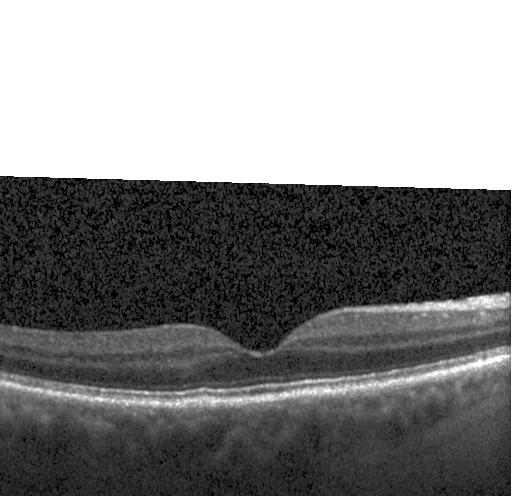
OCT B-scan, macular scan, spectral-domain OCT.
Diagnosis: no choroidal neovascularization, no diabetic macular edema, and no drusen.